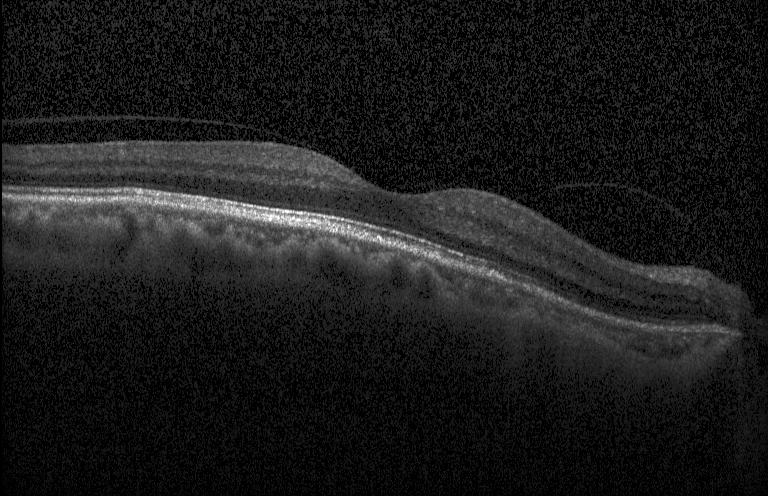 OCT finding: no choroidal neovascularization, diabetic macular edema, or drusen.